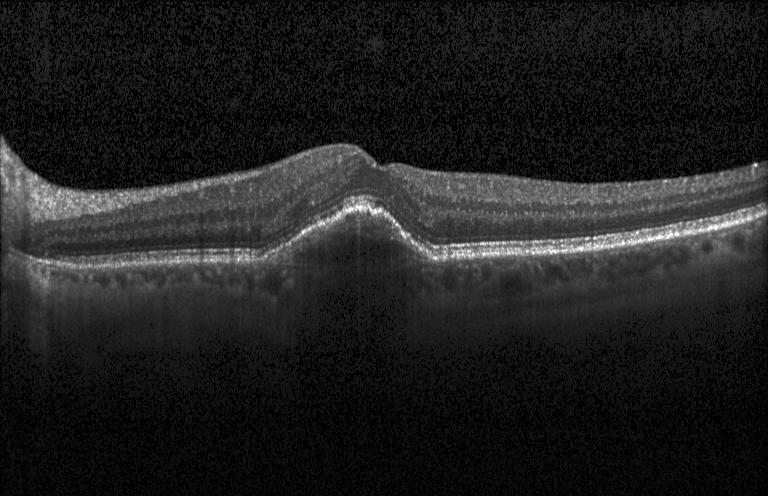 Impression: a choroidal neovascular membrane.